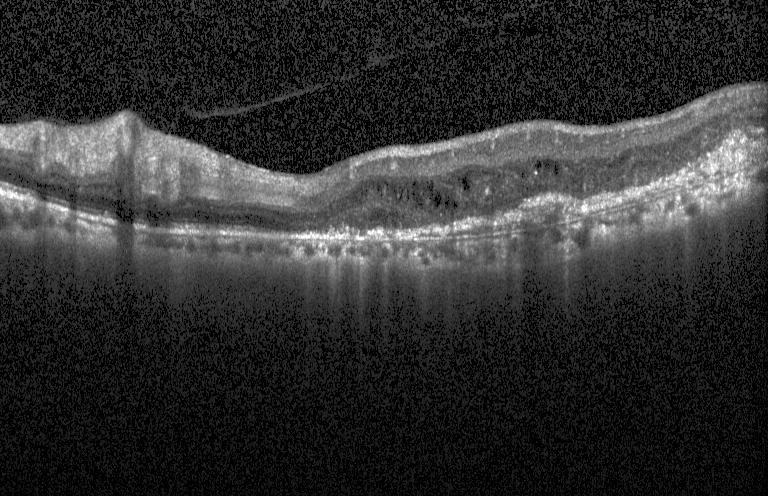

Retinal OCT cross-section.
Choroidal neovascularization (CNV).